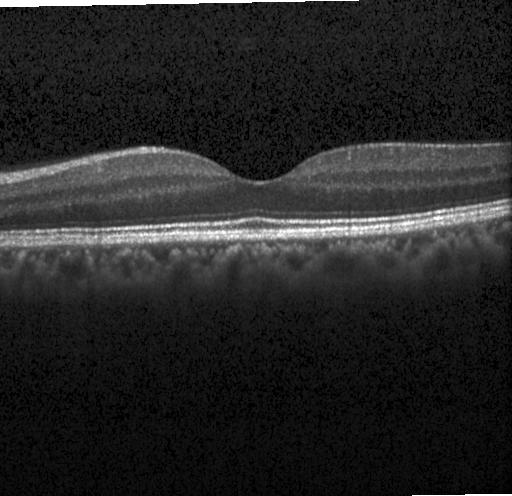 Optical coherence tomography B-scan.
OCT finding: no choroidal neovascularization, no diabetic macular edema, and no drusen.